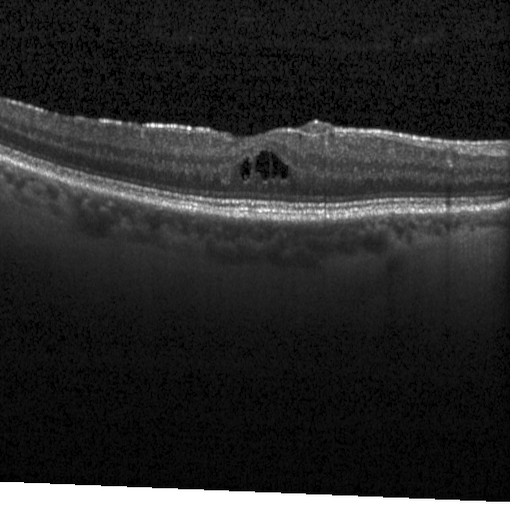

Retinal OCT cross-section — Finding: DME.